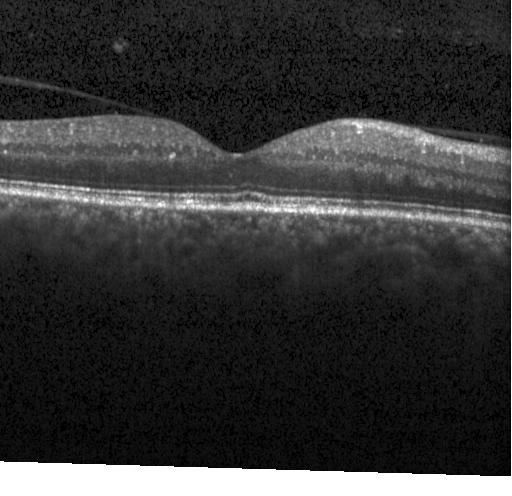

Retinal OCT cross-section
Dx: neither choroidal neovascularization, diabetic macular edema, nor drusen.